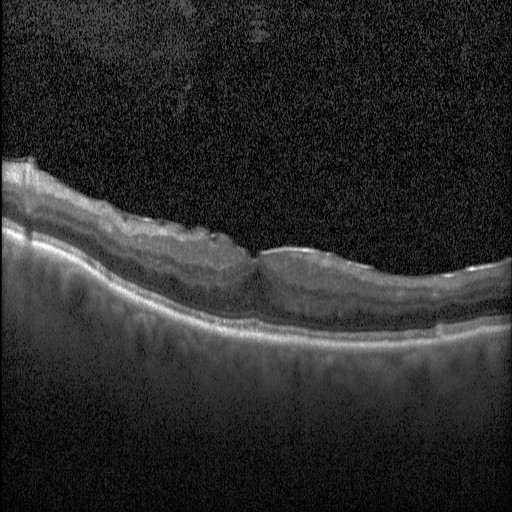 Macular OCT: diabetic macular edema (DME).